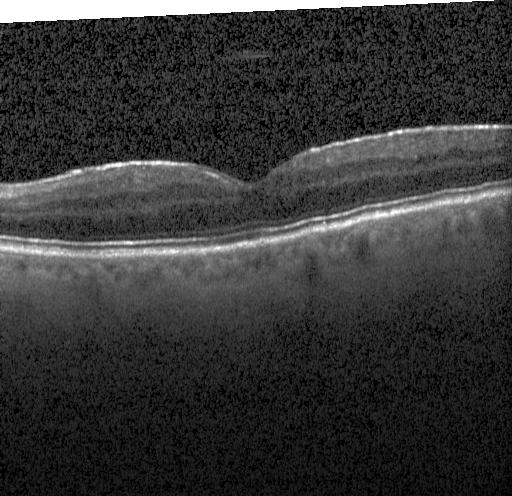
Acquired on a Heidelberg Spectralis. SD-OCT. Macular scan. Retinal OCT B-scan.
Dx: no choroidal neovascularization, diabetic macular edema, or drusen.